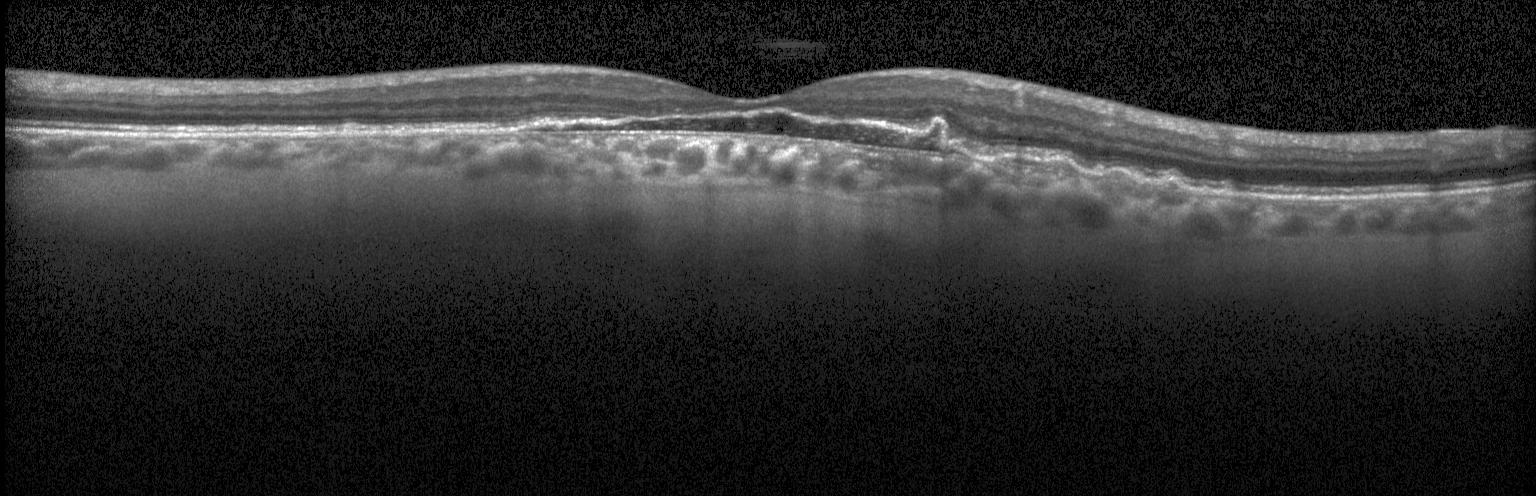 Spectral-domain optical coherence tomography; optical coherence tomography scan.
Choroidal neovascularization.